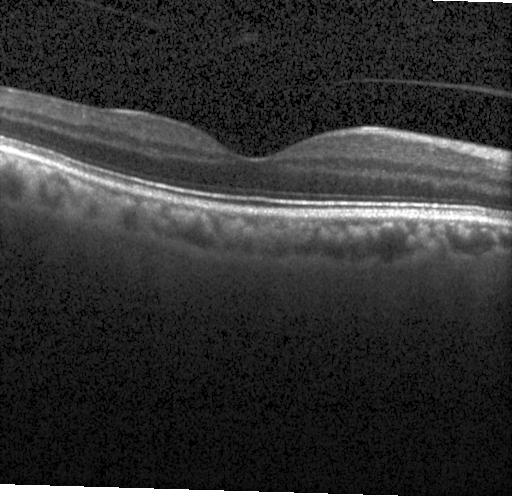
OCT line scan. Macular OCT: neither CNV, DME, nor drusen.